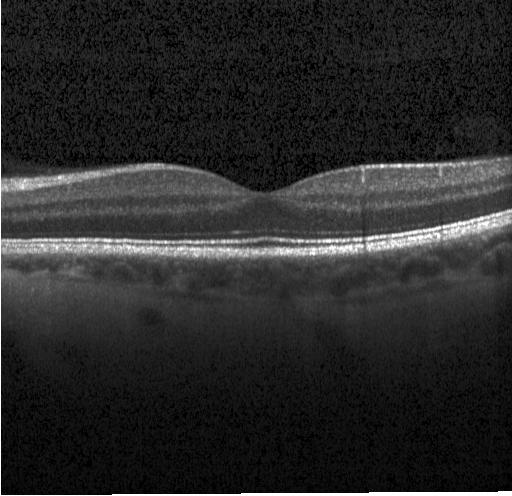 OCT finding: neither choroidal neovascularization, diabetic macular edema, nor drusen.